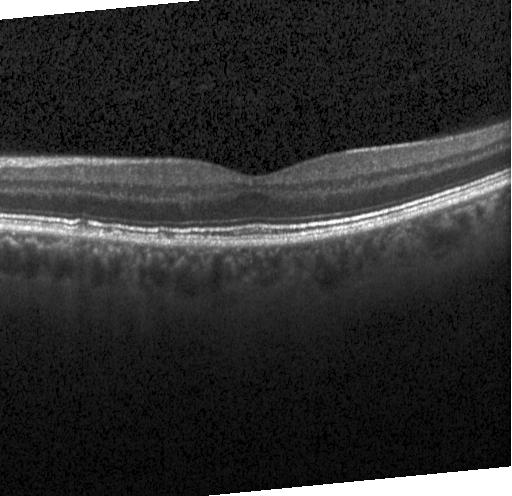
Spectral-domain OCT, horizontal scan through the fovea, acquired on a Heidelberg Spectralis, retinal OCT cross-section — Macular OCT: neither choroidal neovascularization, diabetic macular edema, nor drusen.